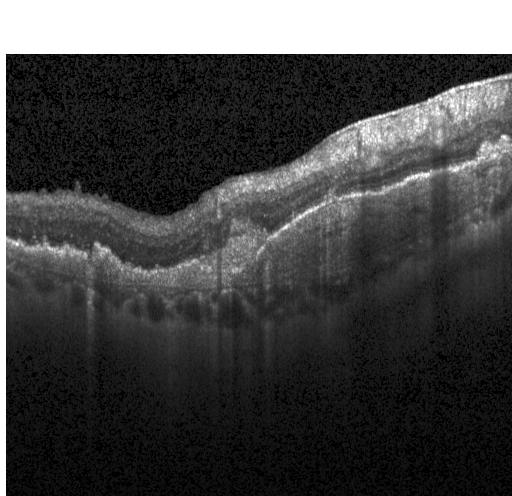 Dx: a choroidal neovascular membrane.